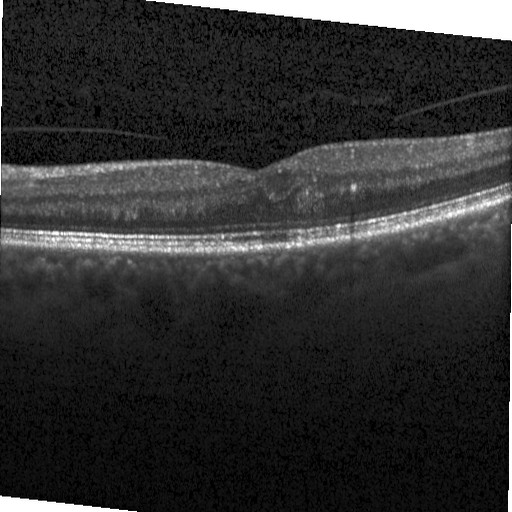 Heidelberg Spectralis; retinal OCT cross-section.
Assessment: diabetic macular edema (DME).